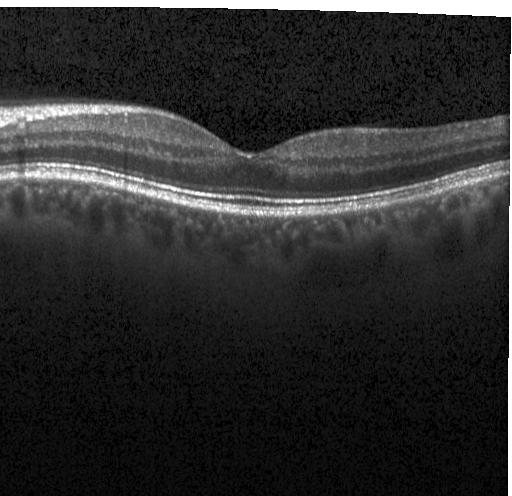

Assessment: no choroidal neovascularization, no diabetic macular edema, and no drusen.